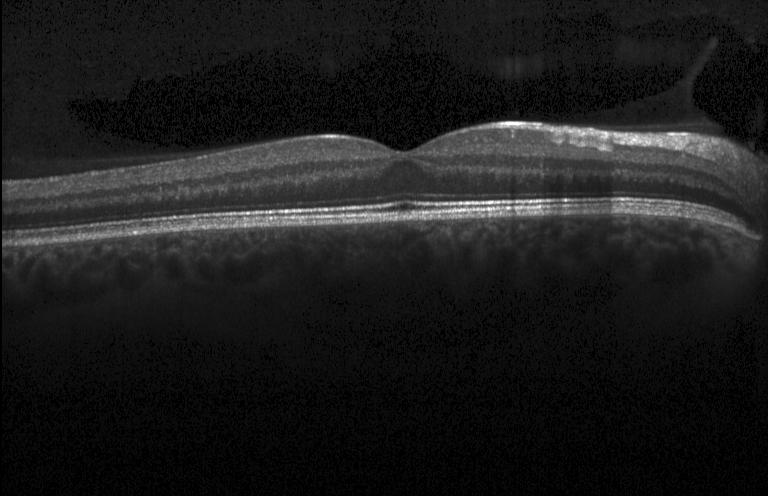 The scan shows neither choroidal neovascularization, diabetic macular edema, nor drusen.